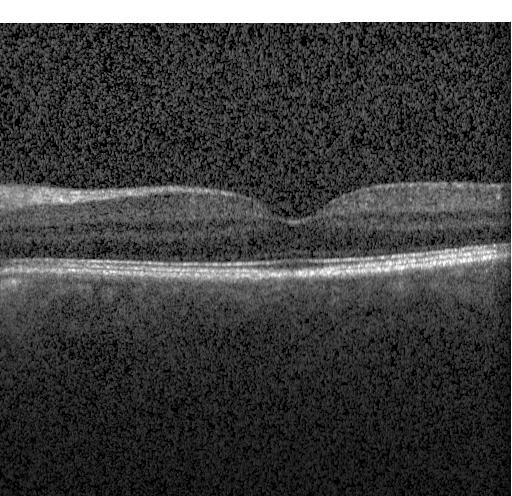

Retinal OCT cross-section showing no evidence of choroidal neovascularization, diabetic macular edema, or drusen.